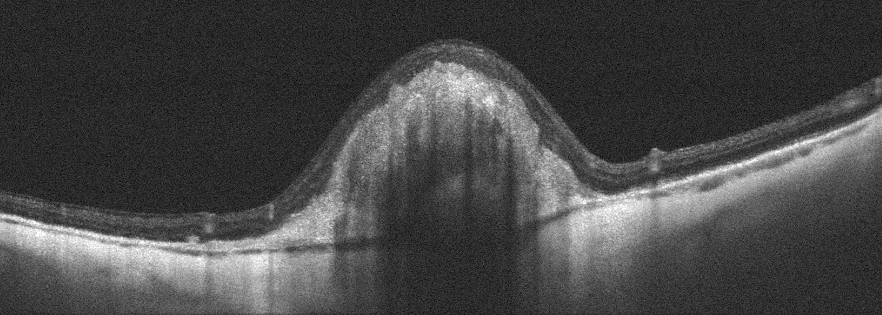 Right eye · optical coherence tomography scan.
Diagnosis: AMD.